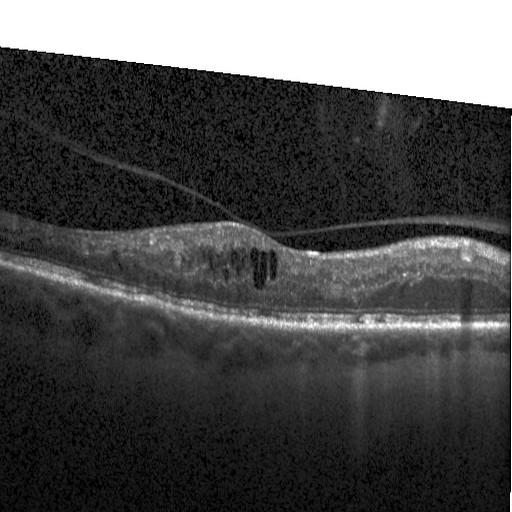
Horizontal scan through the fovea · OCT line scan · spectral-domain OCT — Diagnosis: diabetic macular edema.